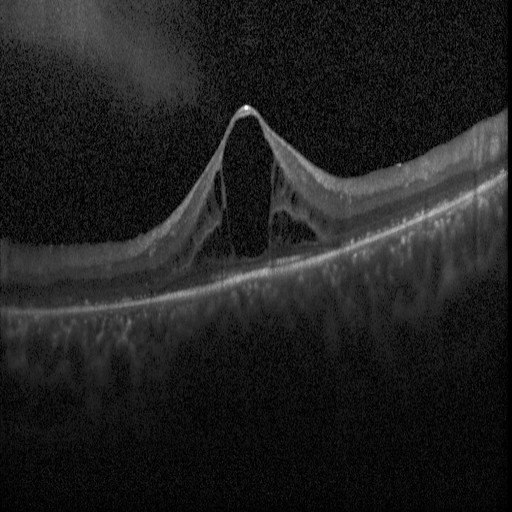

Macular scan. Spectral-domain optical coherence tomography. Optical coherence tomography B-scan
This B-scan demonstrates diabetic macular edema (DME).